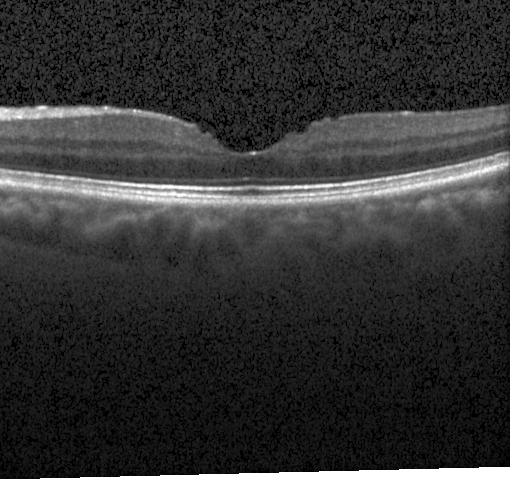
Optical coherence tomography scan · spectral-domain optical coherence tomography
Impression: neither choroidal neovascularization, diabetic macular edema, nor drusen.